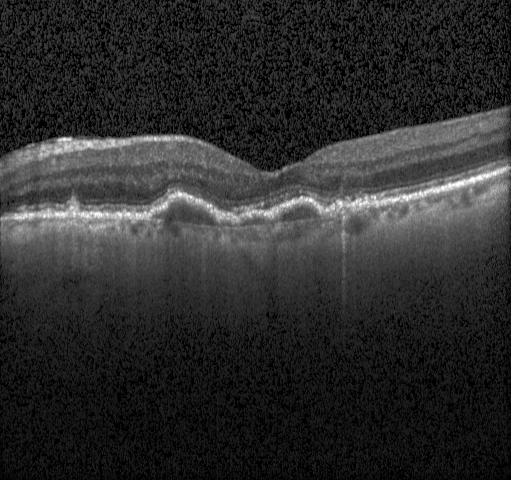

Retinal OCT cross-section. Acquired on a Heidelberg Spectralis.
Diagnosis: CNV.